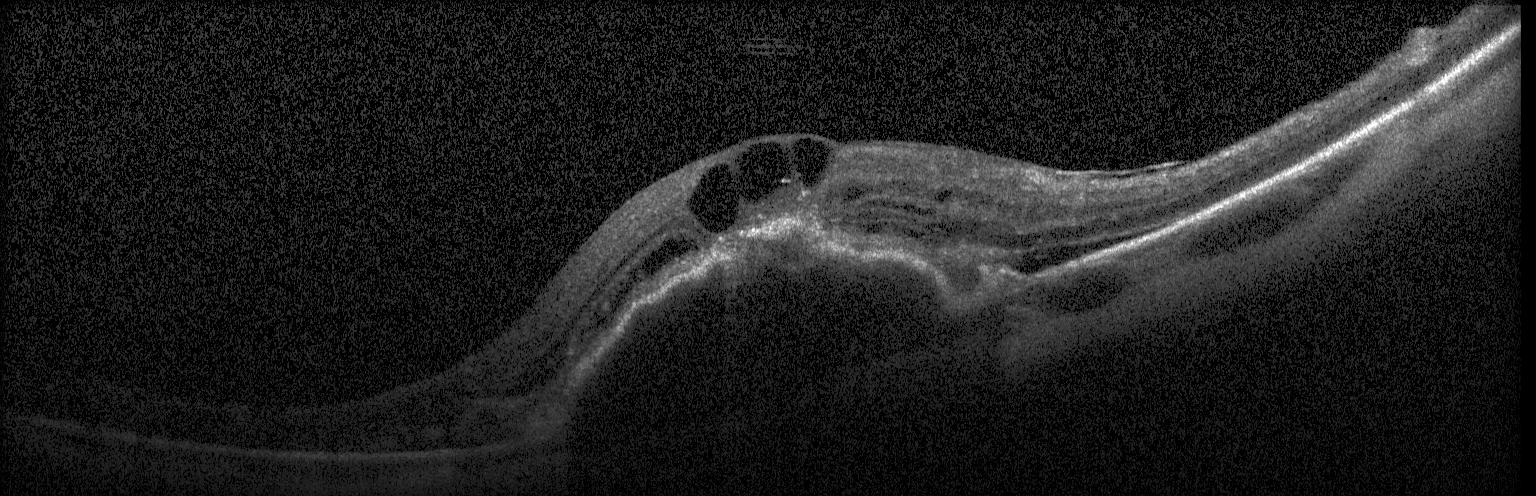

SD-OCT, horizontal scan through the fovea, acquired on a Heidelberg Spectralis, optical coherence tomography scan. Dx: CNV.